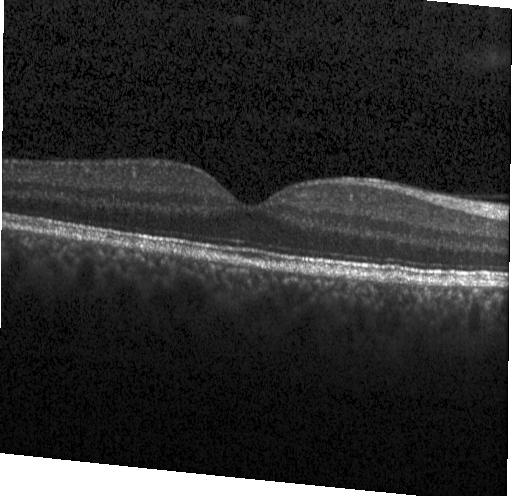 Retinal OCT B-scan; spectral-domain optical coherence tomography
The scan shows no evidence of choroidal neovascularization, diabetic macular edema, or drusen.